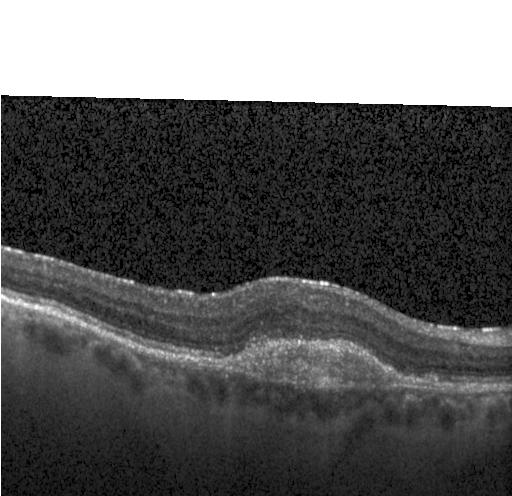
Retinal OCT cross-section
Diagnosis: a choroidal neovascular membrane.